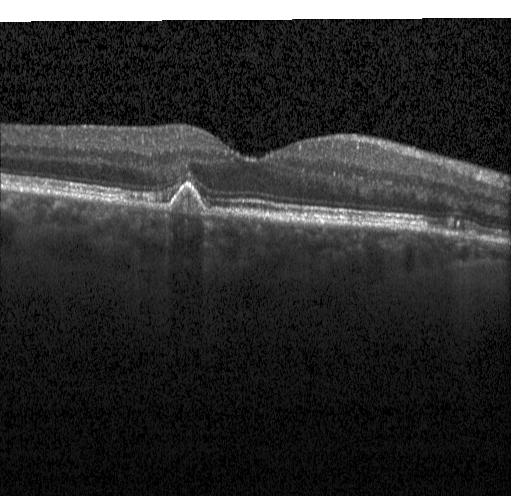

Diagnosis: sub-RPE drusenoid deposits.